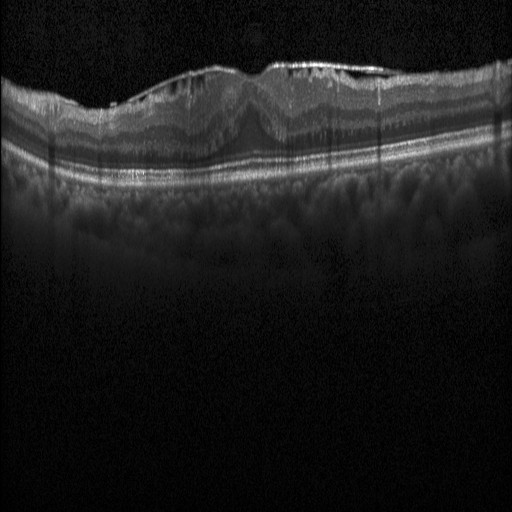

Diagnosis: diabetic macular edema (DME).